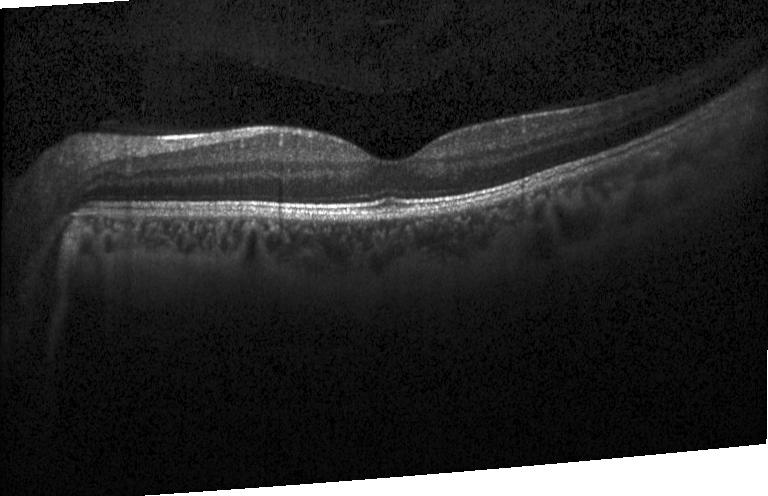
Macular scan; optical coherence tomography B-scan; SD-OCT; instrument: Heidelberg Spectralis — This B-scan demonstrates no choroidal neovascularization, diabetic macular edema, or drusen.